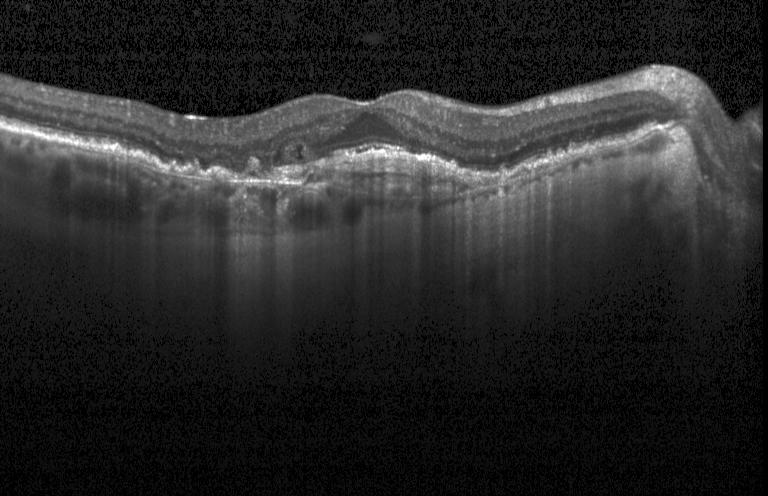
Optical coherence tomography B-scan
Diagnosis: choroidal neovascularization (CNV).